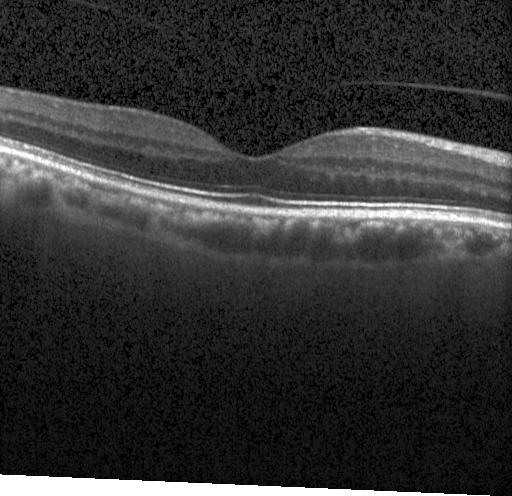 OCT B-scan, spectral-domain OCT, Heidelberg Spectralis — Assessment: neither CNV, DME, nor drusen.